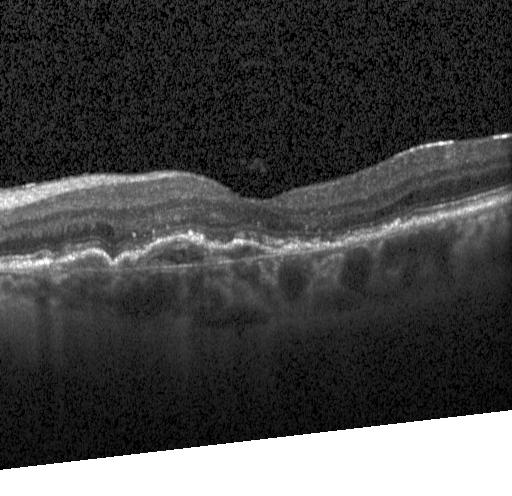

Spectral-domain optical coherence tomography. Horizontal scan through the fovea. OCT line scan. Acquired on a Heidelberg Spectralis
This B-scan demonstrates CNV.